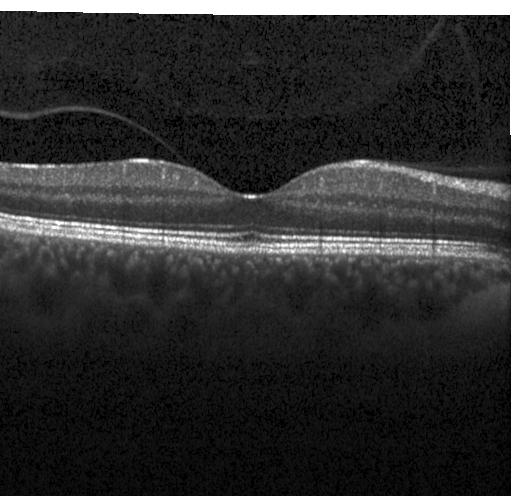 Instrument: Heidelberg Spectralis · retinal OCT cross-section · macular scan
OCT finding: no choroidal neovascularization, no diabetic macular edema, and no drusen.